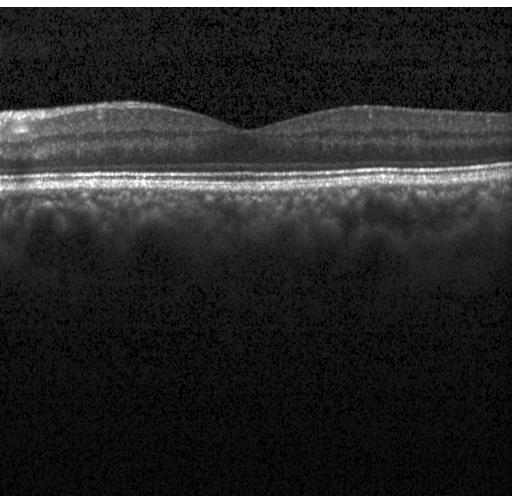 Retinal OCT B-scan; instrument: Heidelberg Spectralis; horizontal scan through the fovea.
The scan shows no evidence of choroidal neovascularization, diabetic macular edema, or drusen.